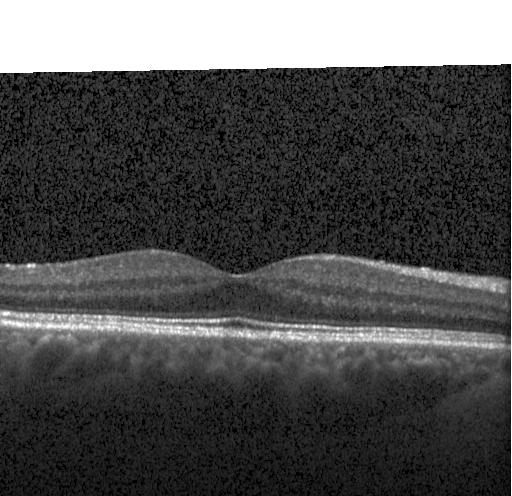
Retinal OCT cross-section, Heidelberg Spectralis, macular scan, spectral-domain OCT.
Impression: neither choroidal neovascularization, diabetic macular edema, nor drusen.